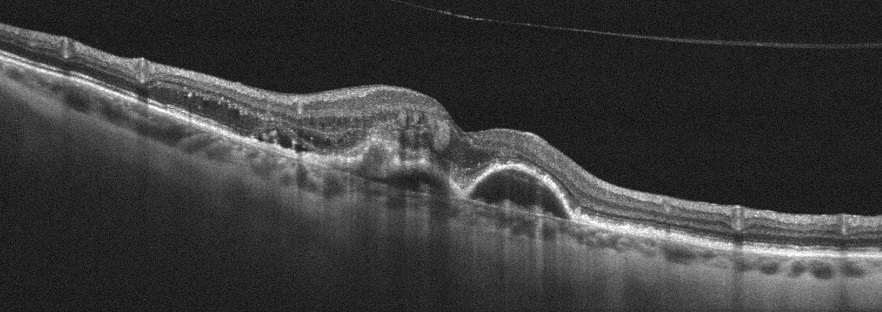

Macular OCT: age-related macular degeneration.